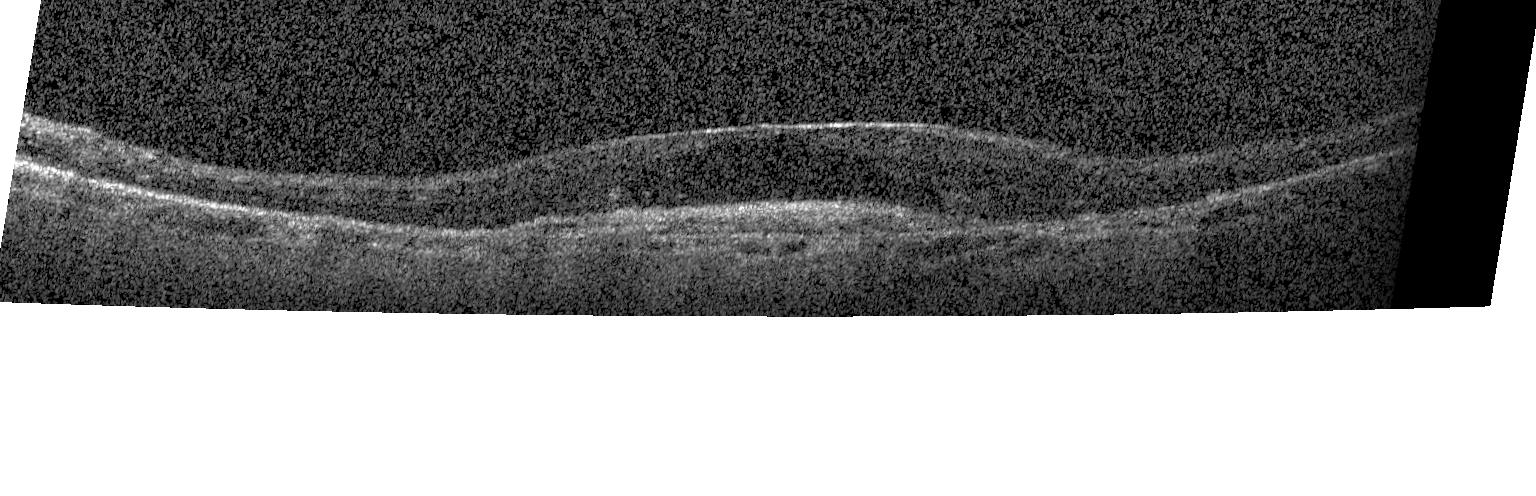

Spectral-domain OCT B-scan: choroidal neovascularization (CNV).